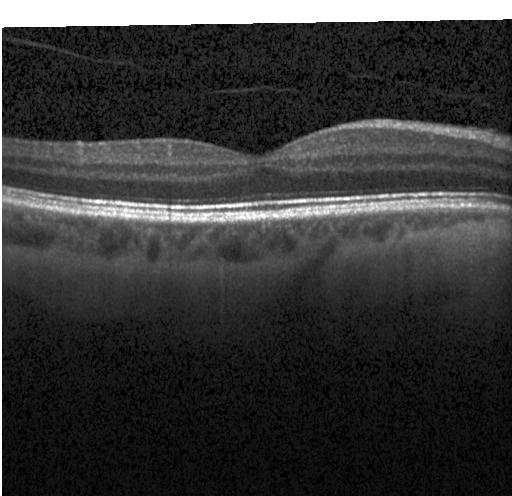 Acquired on a Heidelberg Spectralis. Through the macula. OCT B-scan — Diagnosis: no CNV, DME, or drusen.